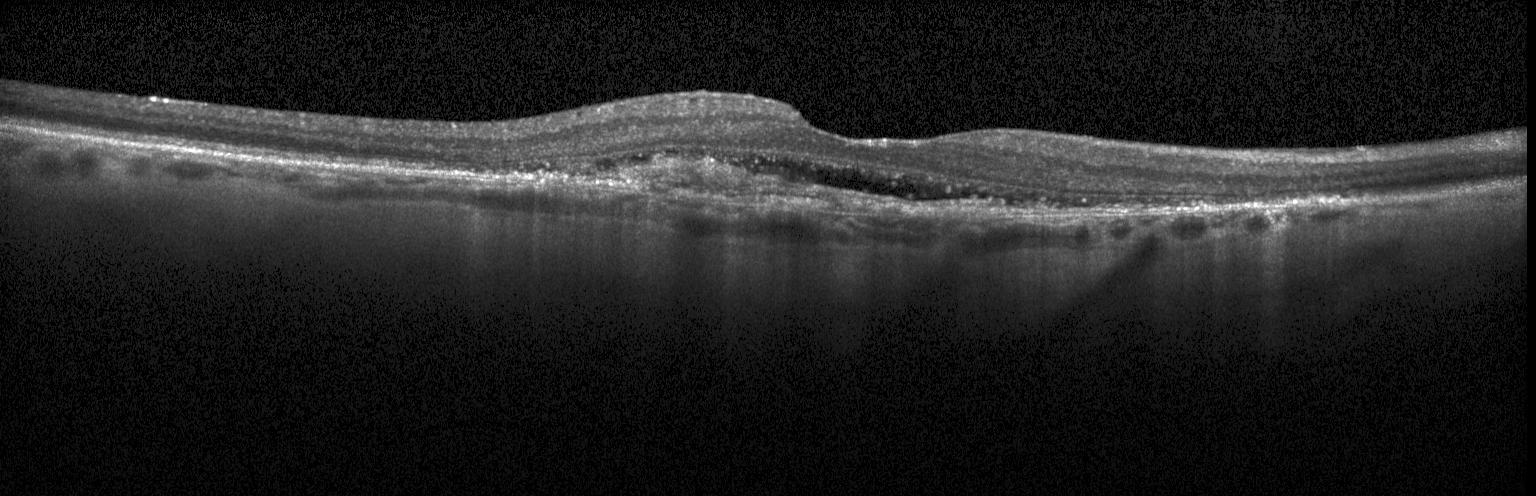 SD-OCT · through the macula · Heidelberg Spectralis · retinal OCT B-scan — Dx: CNV.